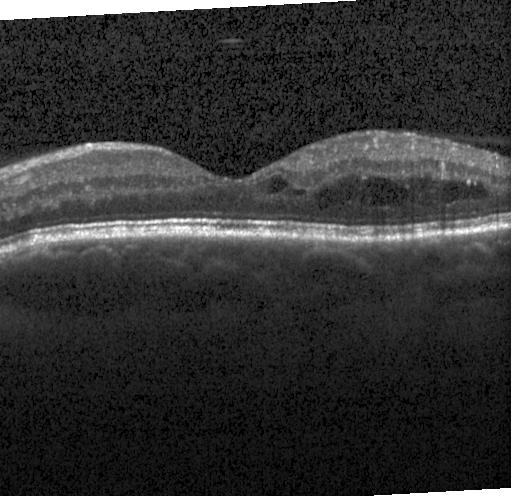
Impression: diabetic macular edema (DME).